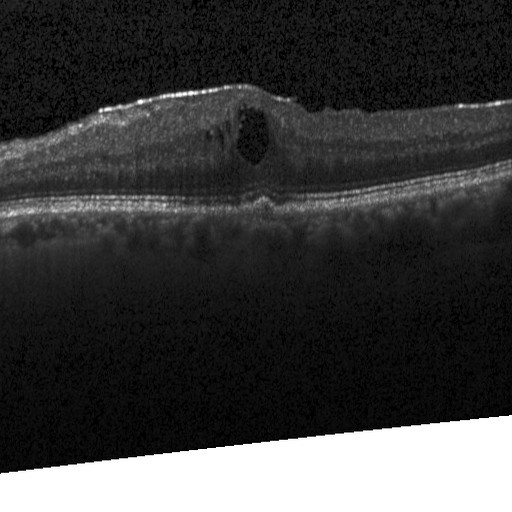

The scan shows diabetic macular edema.